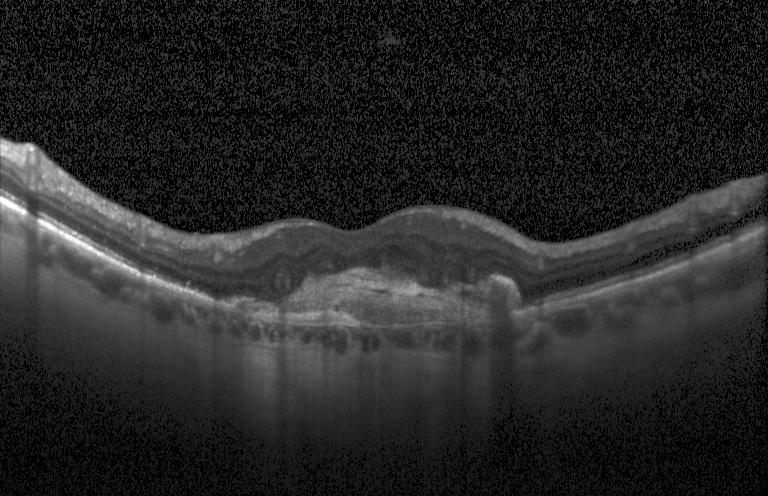 Centered on the fovea; OCT line scan; instrument: Heidelberg Spectralis.
Assessment: a choroidal neovascular membrane.